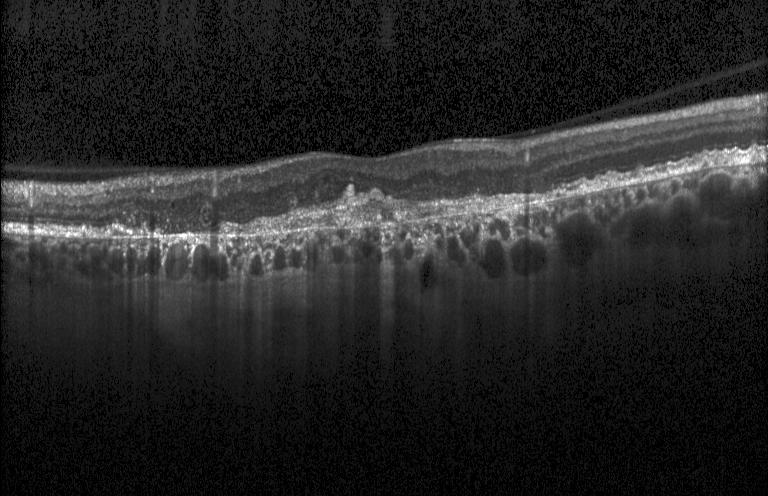
Acquired on a Heidelberg Spectralis. OCT B-scan. Spectral-domain OCT. Centered on the fovea.
OCT finding: choroidal neovascularization (CNV).